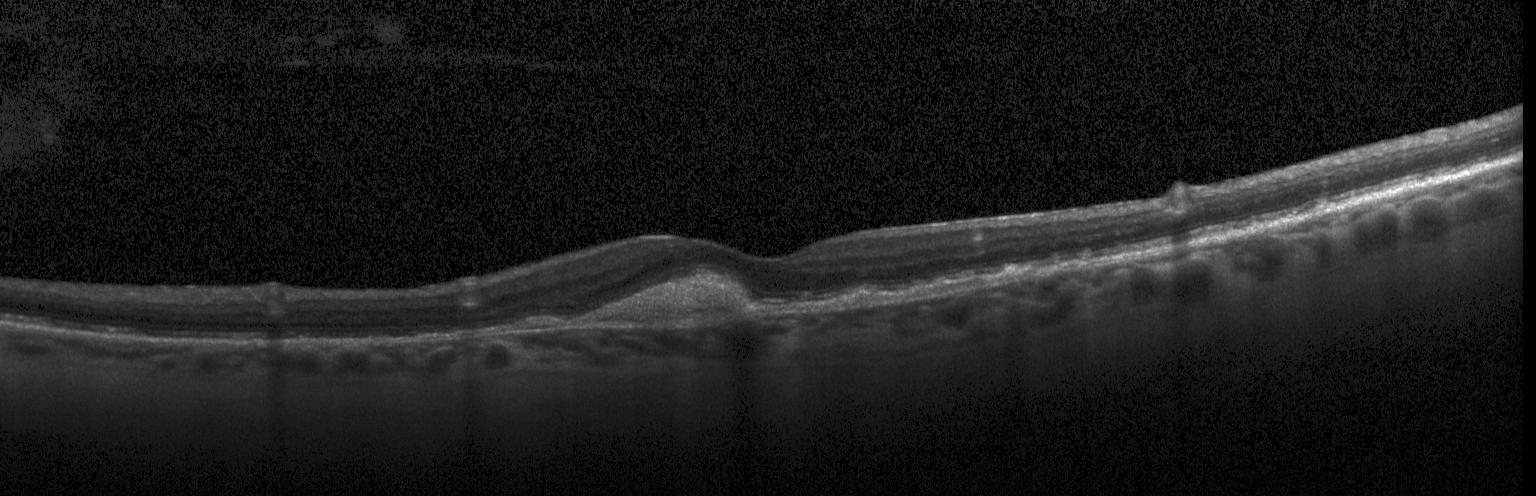 Diagnosis: a choroidal neovascular membrane.